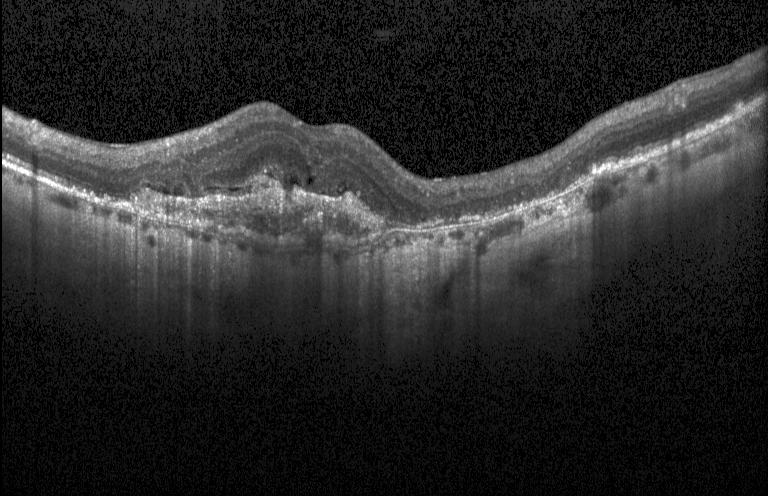
Diagnosis: a choroidal neovascular membrane.